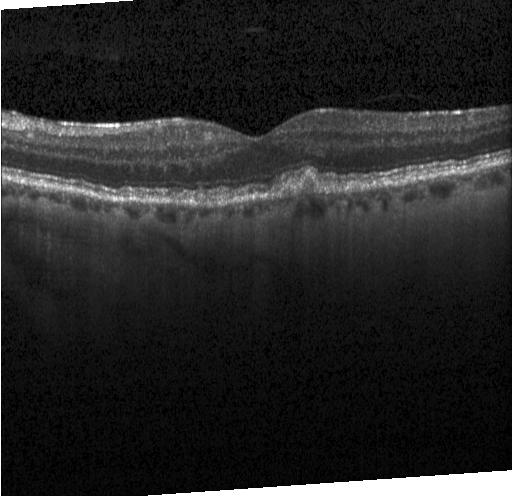

Retinal OCT B-scan.
Diagnosis: drusen.